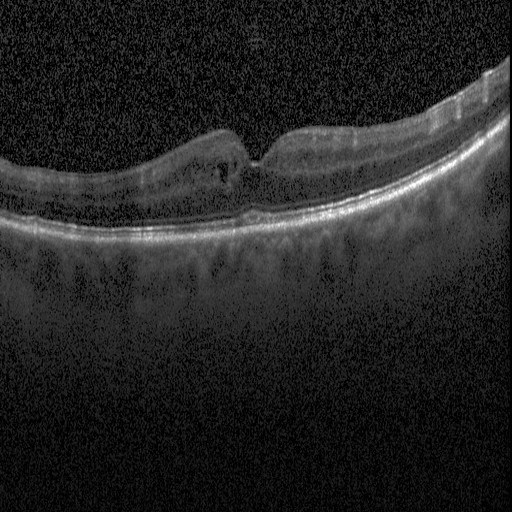

Retinal OCT cross-section
The scan shows diabetic macular edema.